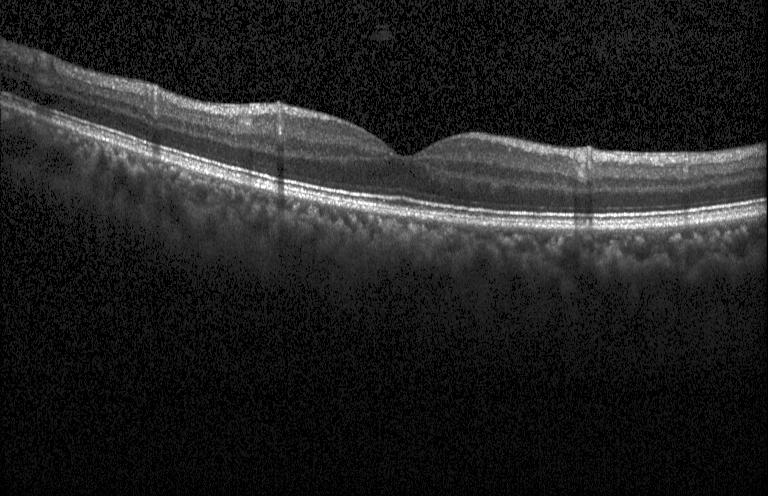 OCT B-scan — No choroidal neovascularization, diabetic macular edema, or drusen.